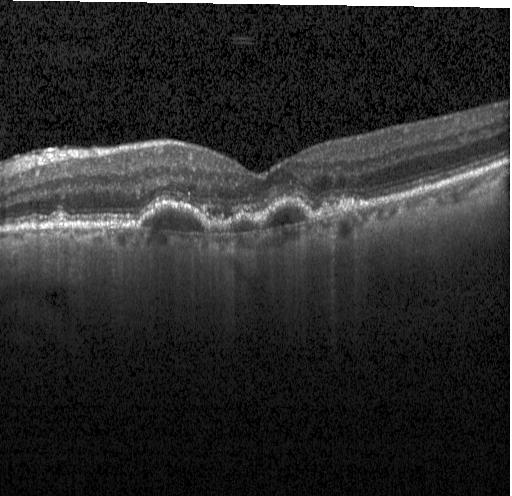
Spectral-domain OCT. Heidelberg Spectralis OCT system. Optical coherence tomography B-scan. Through the macula. OCT finding: choroidal neovascularization.